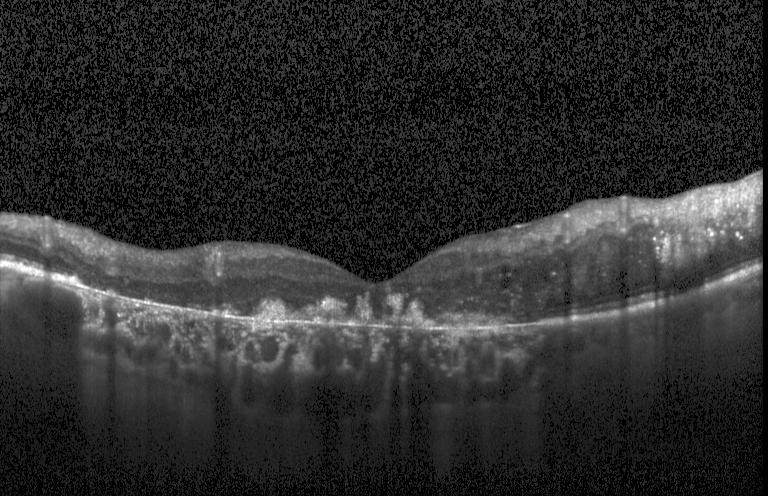
Optical coherence tomography B-scan.
Macular OCT: a choroidal neovascular membrane.